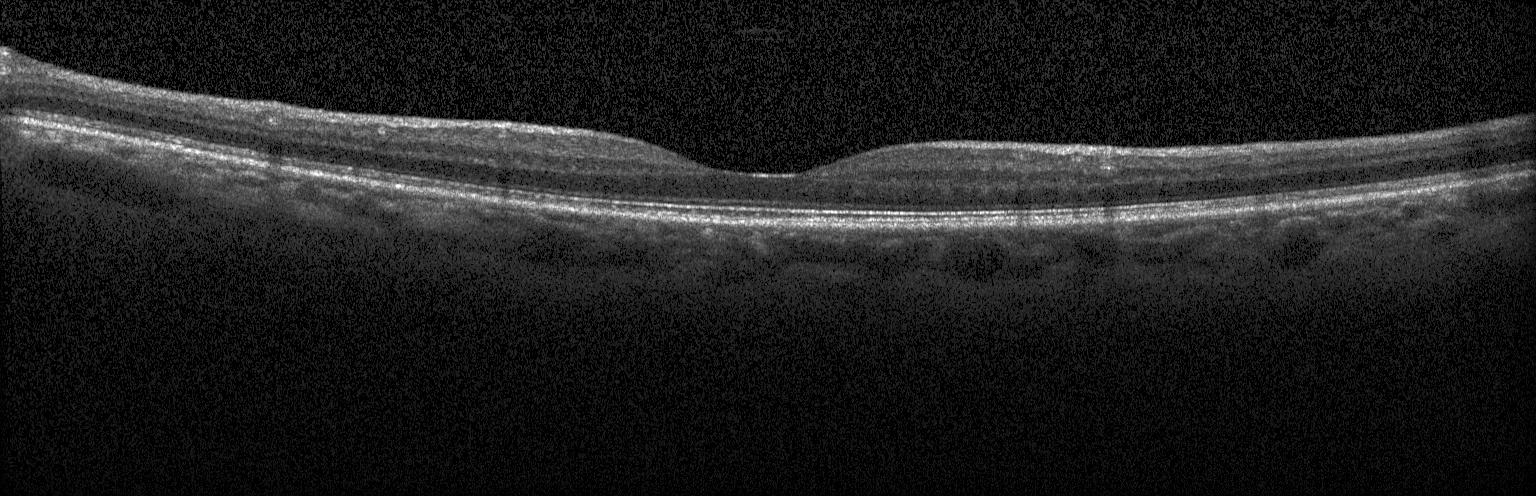
Retinal OCT cross-section
OCT finding: no choroidal neovascularization, diabetic macular edema, or drusen.